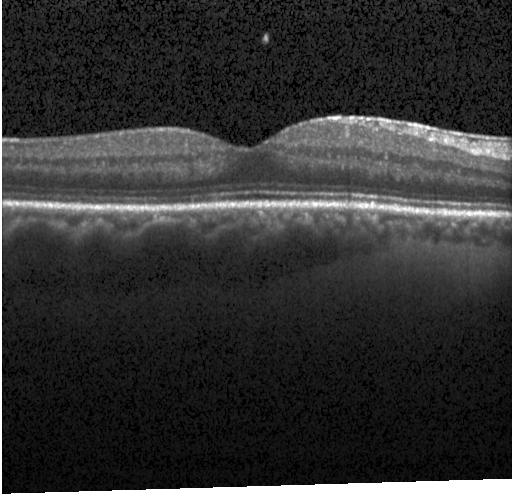
Optical coherence tomography B-scan; SD-OCT.
Dx: no evidence of choroidal neovascularization, diabetic macular edema, or drusen.